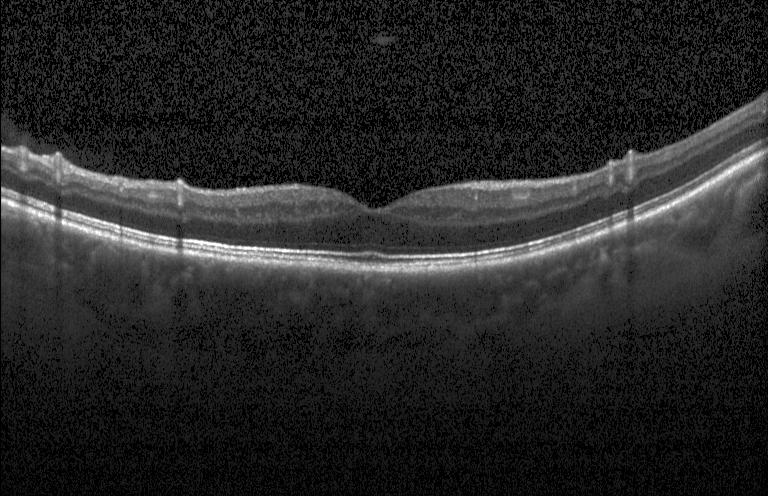 Heidelberg Spectralis OCT system; macular scan; SD-OCT; optical coherence tomography scan — Diagnosis: no choroidal neovascularization, diabetic macular edema, or drusen.